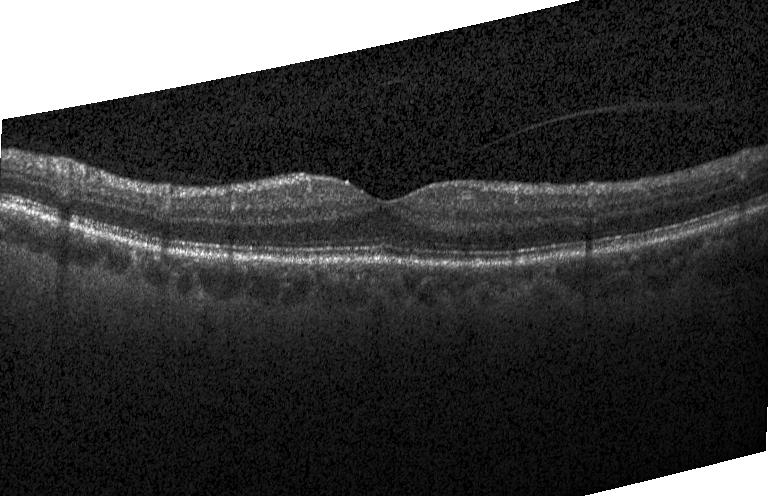

OCT B-scan showing neither choroidal neovascularization, diabetic macular edema, nor drusen.